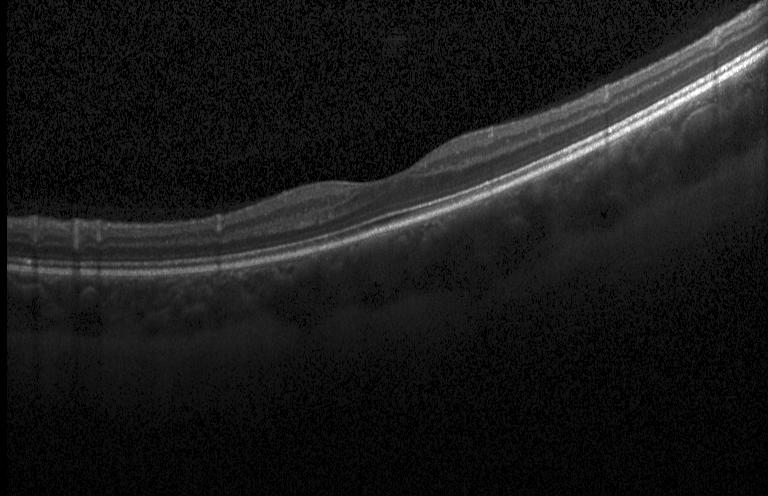 Optical coherence tomography B-scan
Dx: no evidence of CNV, DME, or drusen.